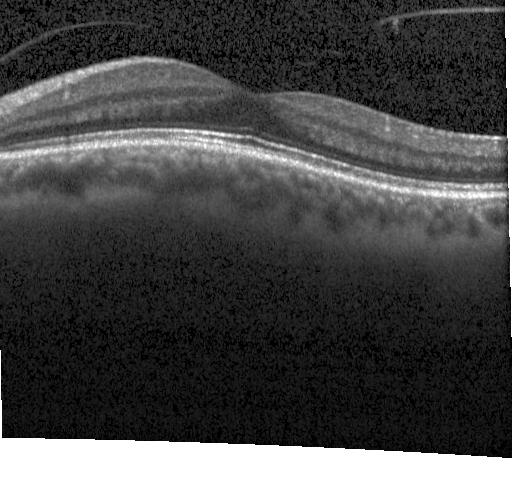
Finding: no choroidal neovascularization, diabetic macular edema, or drusen.